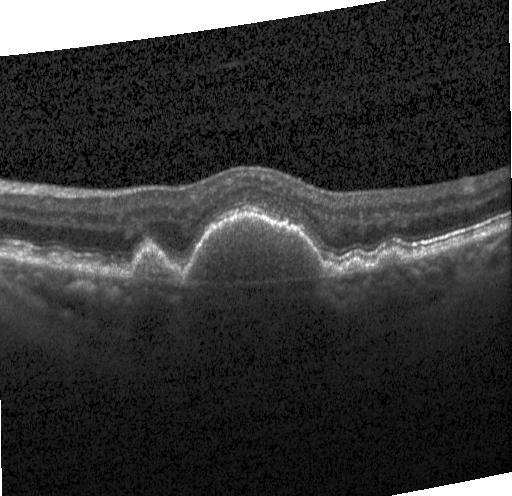

Macular scan, acquired on a Heidelberg Spectralis, SD-OCT, OCT line scan. A choroidal neovascular membrane.